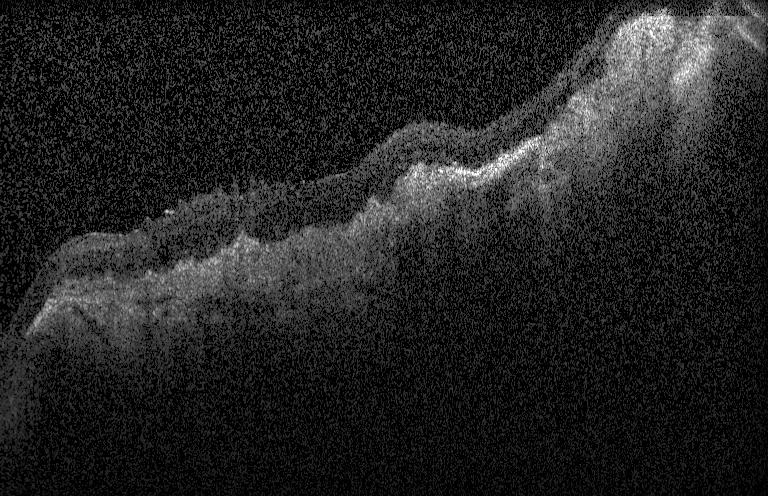
Through the macula, instrument: Heidelberg Spectralis, OCT line scan. CNV.